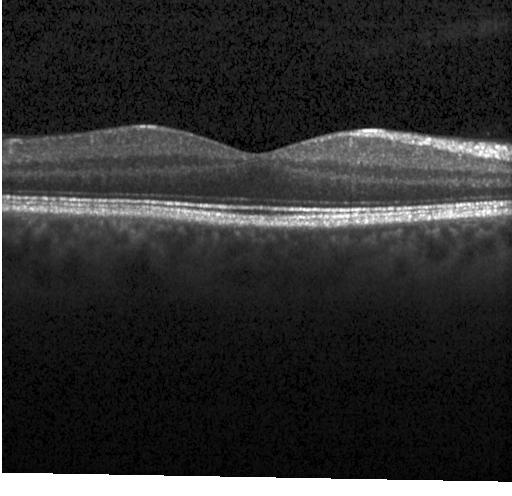 Assessment: no choroidal neovascularization, no diabetic macular edema, and no drusen.